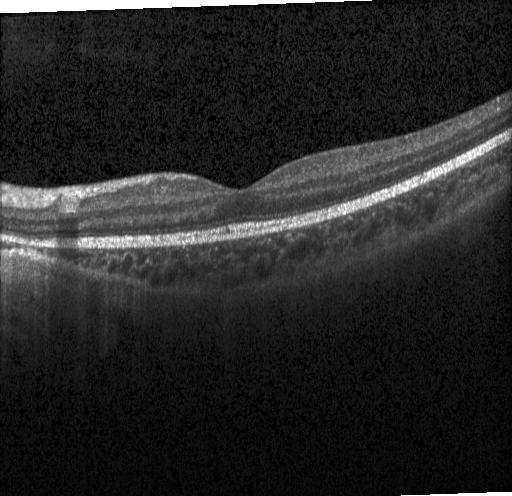
Retinal OCT cross-section showing no evidence of choroidal neovascularization, diabetic macular edema, or drusen.